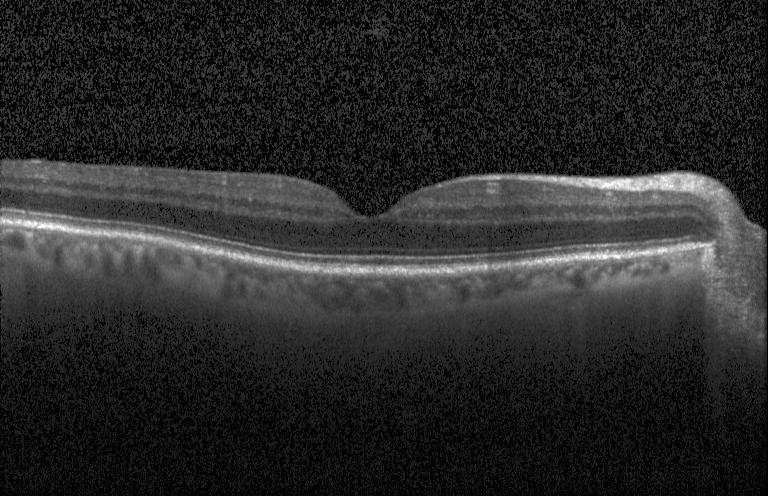 OCT line scan
Assessment: no choroidal neovascularization, diabetic macular edema, or drusen.